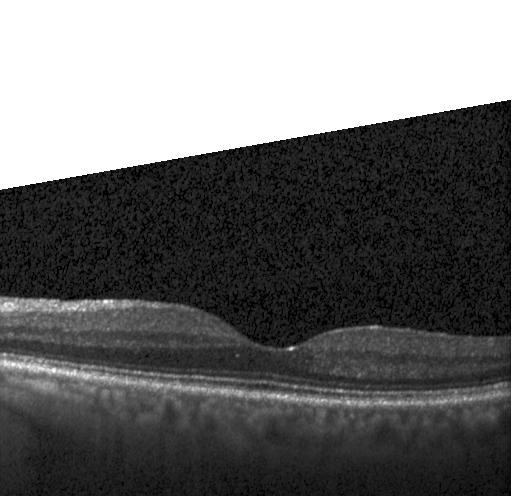
Diagnosis: no choroidal neovascularization, no diabetic macular edema, and no drusen.